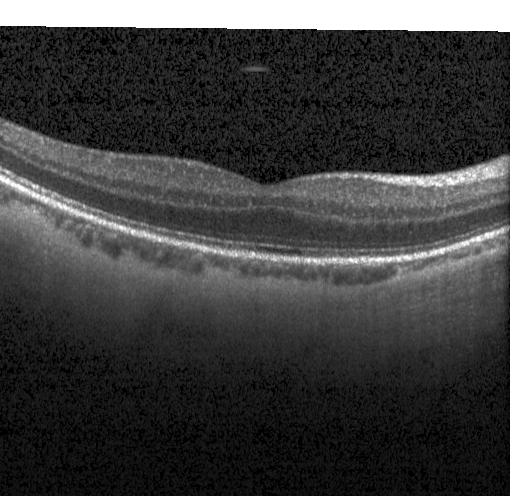

Macular OCT demonstrating no evidence of choroidal neovascularization, diabetic macular edema, or drusen.